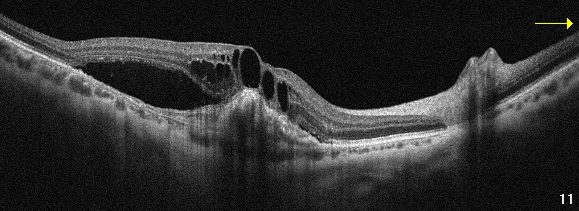
Right eye · optical coherence tomography scan — Finding: AMD.